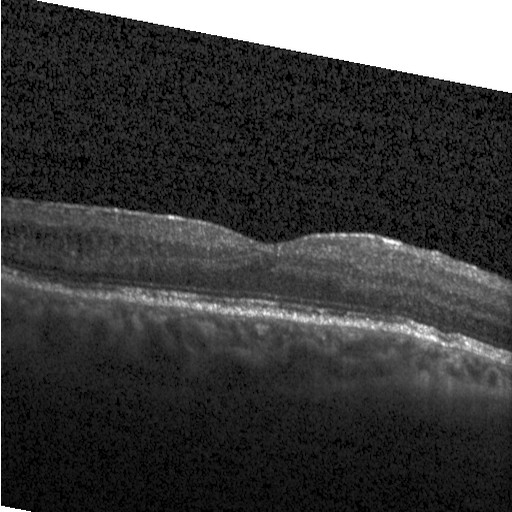 Finding: diabetic macular edema (DME).